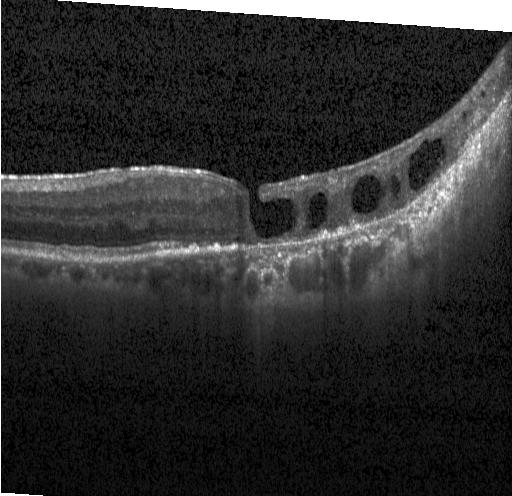 Retinal OCT cross-section.
Macular OCT: diabetic macular edema (DME).